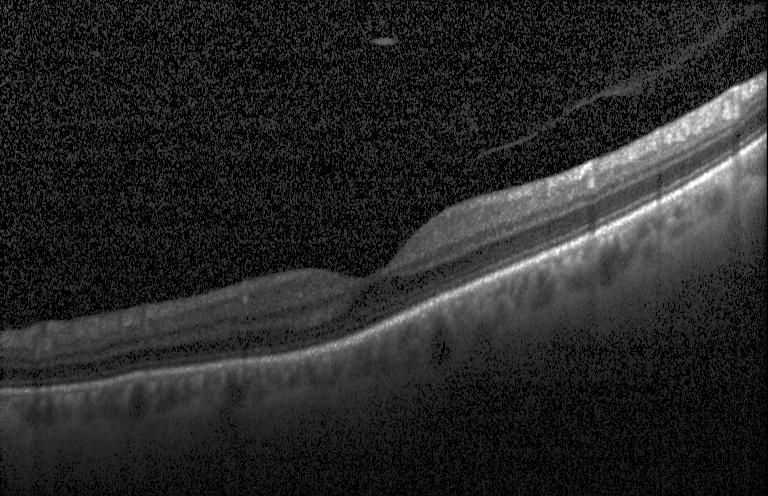 OCT B-scan showing neither CNV, DME, nor drusen.